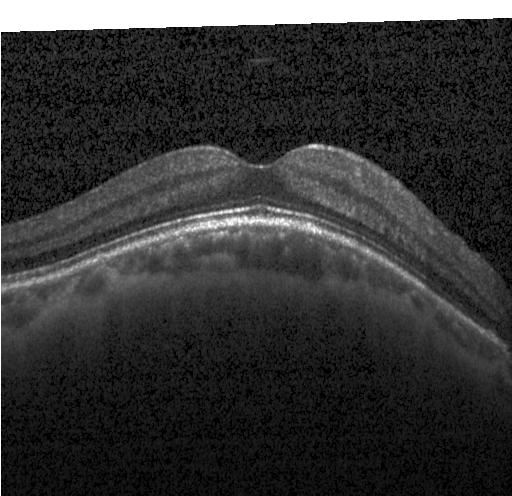 Optical coherence tomography B-scan
OCT finding: no evidence of choroidal neovascularization, diabetic macular edema, or drusen.